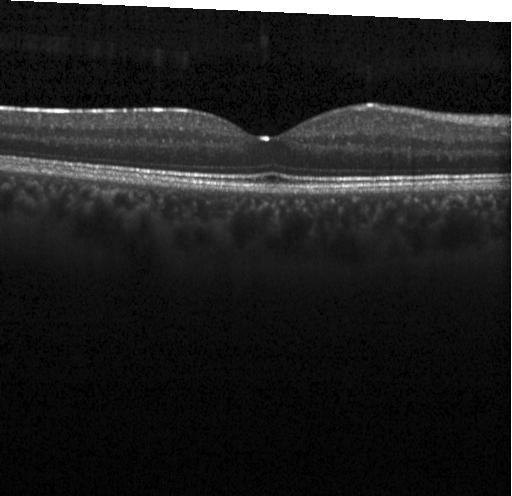

Retinal OCT cross-section showing no choroidal neovascularization, no diabetic macular edema, and no drusen.